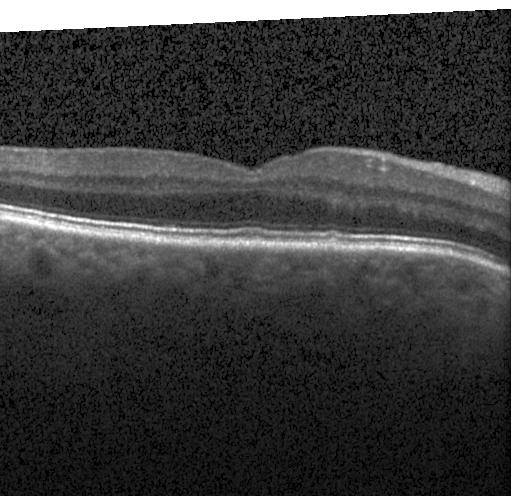
Optical coherence tomography scan. Macular scan. SD-OCT. Heidelberg Spectralis
Macular OCT: no evidence of choroidal neovascularization, diabetic macular edema, or drusen.